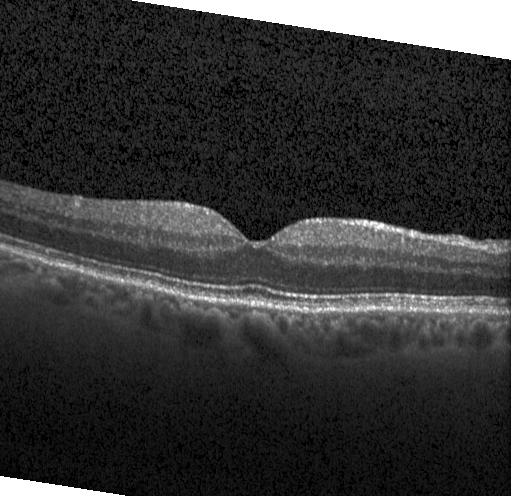

Finding: no evidence of CNV, DME, or drusen.